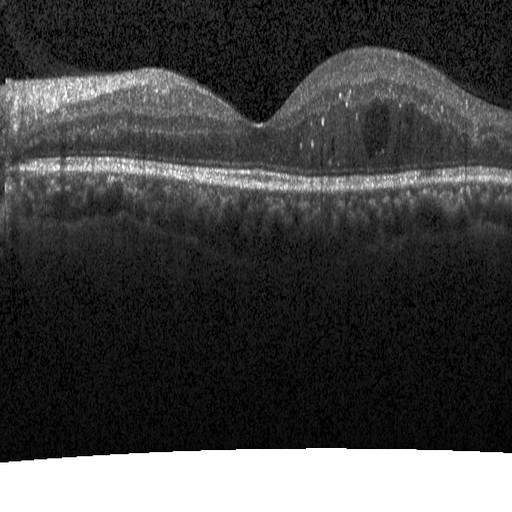

Fovea-centered; spectral-domain optical coherence tomography; instrument: Heidelberg Spectralis; OCT B-scan.
This B-scan demonstrates diabetic macular edema.